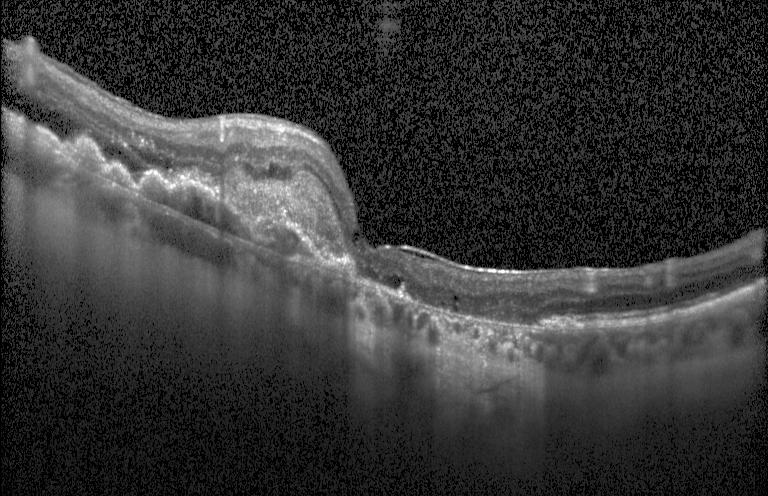
Impression: a choroidal neovascular membrane.